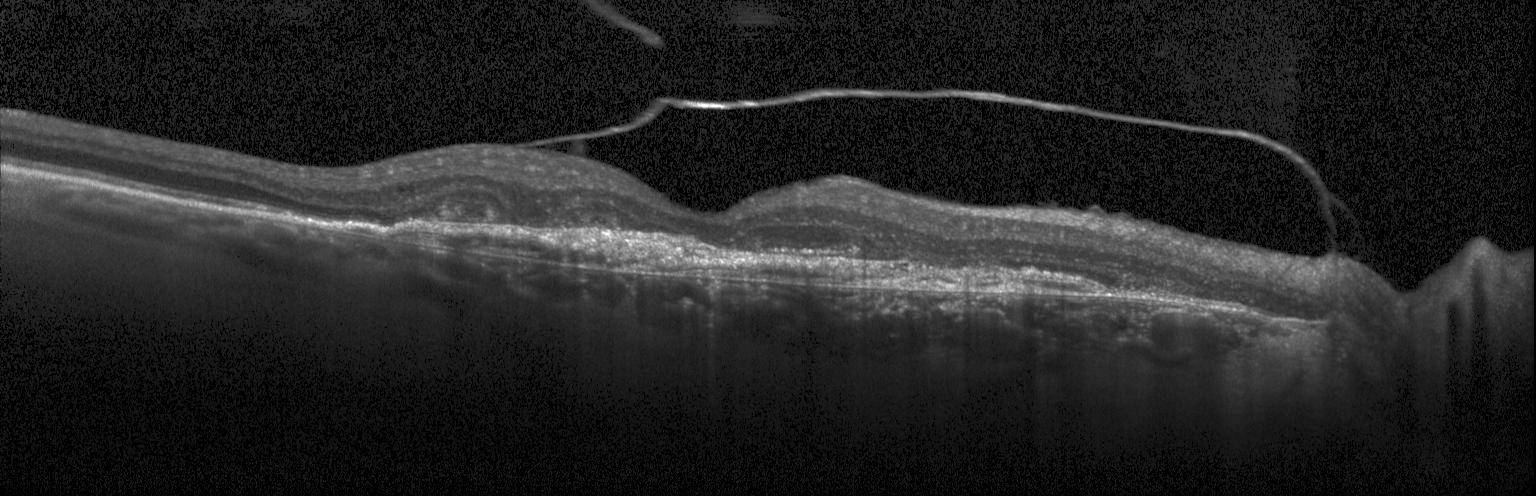
Horizontal scan through the fovea; instrument: Heidelberg Spectralis; OCT B-scan.
The scan shows a choroidal neovascular membrane.